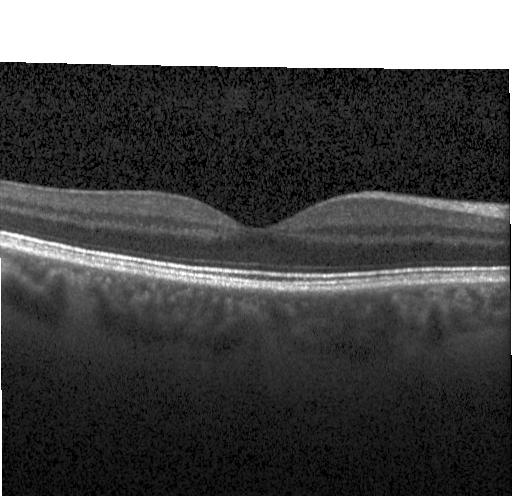

Finding: no choroidal neovascularization, diabetic macular edema, or drusen.